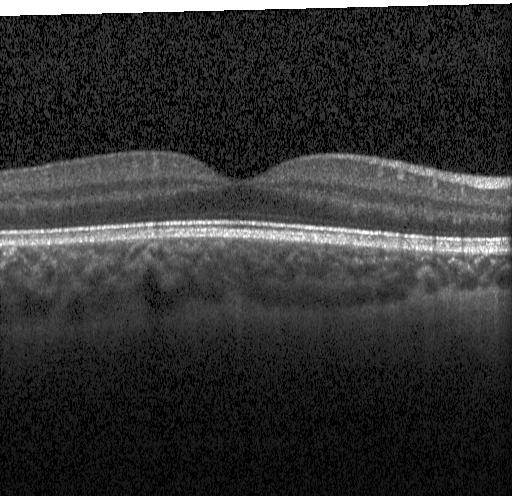 Macular OCT demonstrating neither choroidal neovascularization, diabetic macular edema, nor drusen.